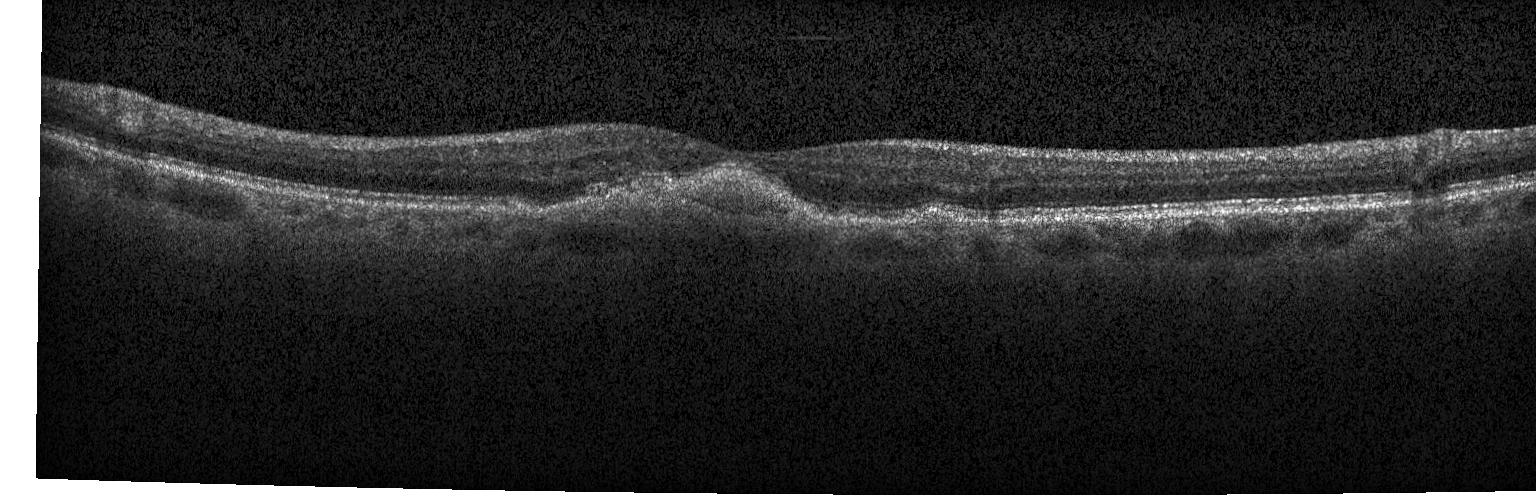 Optical coherence tomography B-scan; spectral-domain optical coherence tomography; Heidelberg Spectralis OCT system; through the macula. A choroidal neovascular membrane.